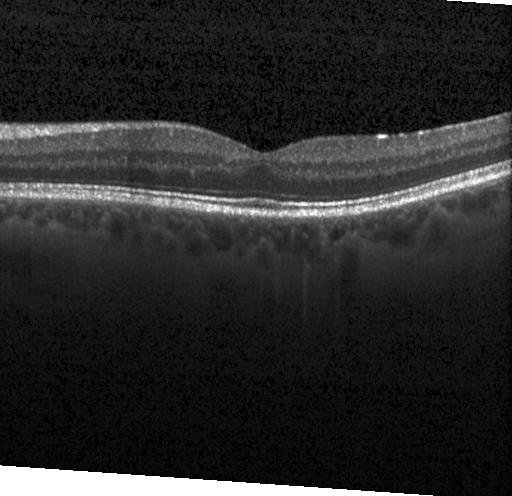

Optical coherence tomography B-scan; acquired on a Heidelberg Spectralis
Diagnosis: no evidence of CNV, DME, or drusen.